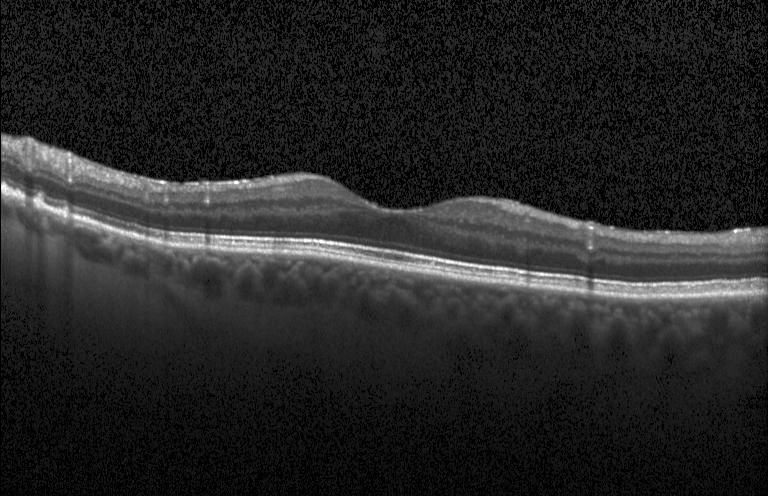

Assessment: no evidence of CNV, DME, or drusen.